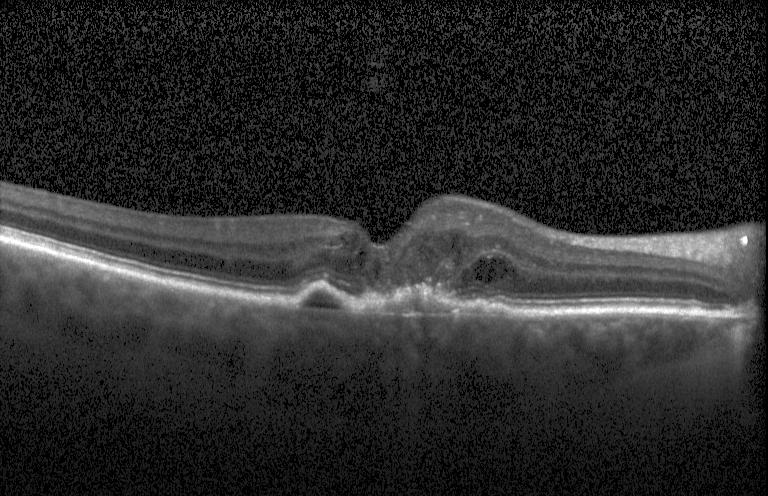 Macular OCT: a choroidal neovascular membrane.